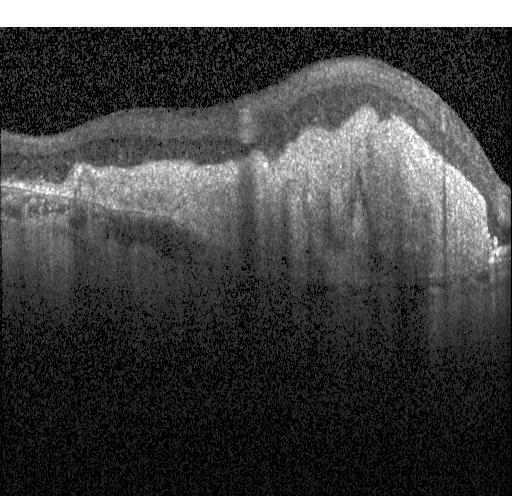 Retinal OCT cross-section; macular scan; Heidelberg Spectralis OCT system. Diagnosis: choroidal neovascularization (CNV).